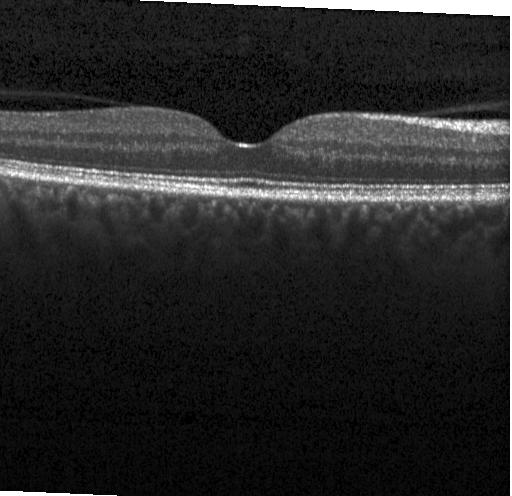

Optical coherence tomography scan.
This B-scan demonstrates no choroidal neovascularization, diabetic macular edema, or drusen.